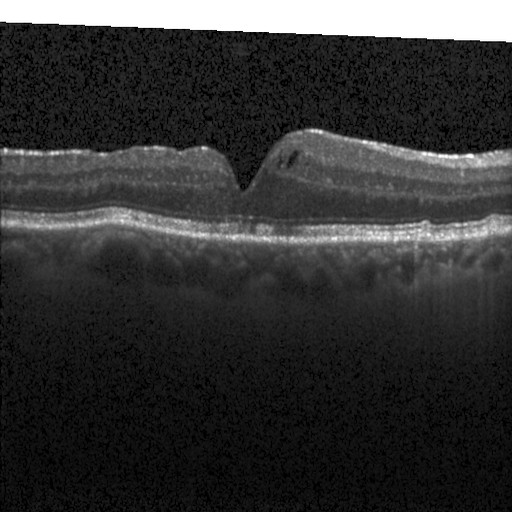

OCT line scan; horizontal scan through the fovea; spectral-domain OCT — Finding: diabetic macular edema.